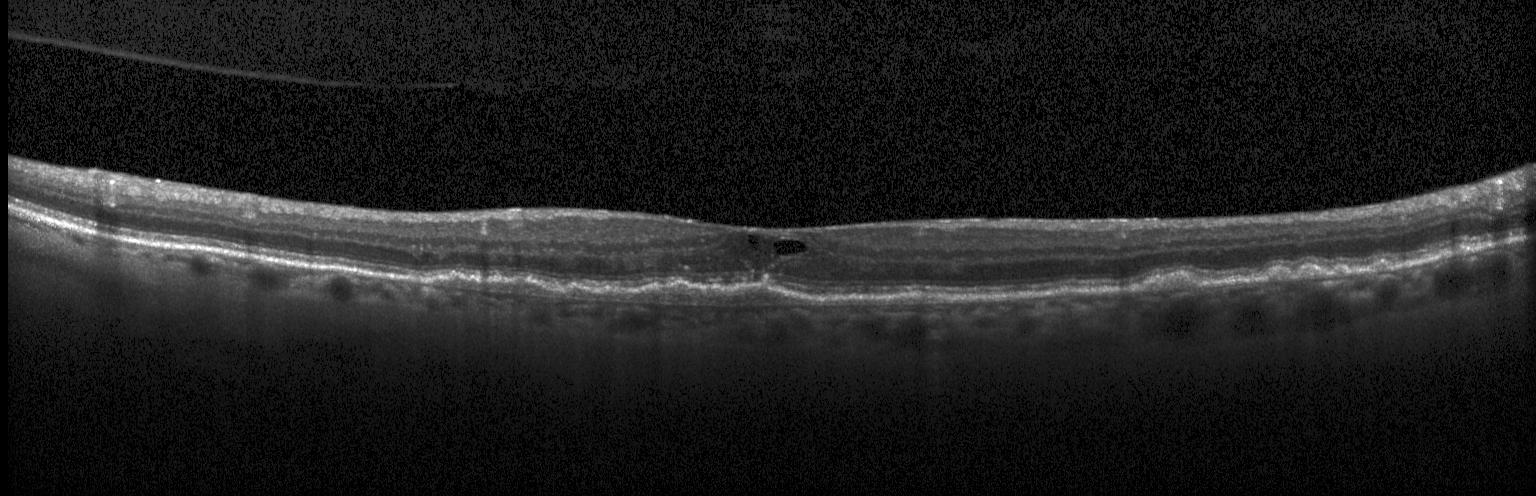

OCT line scan — Finding: a choroidal neovascular membrane.